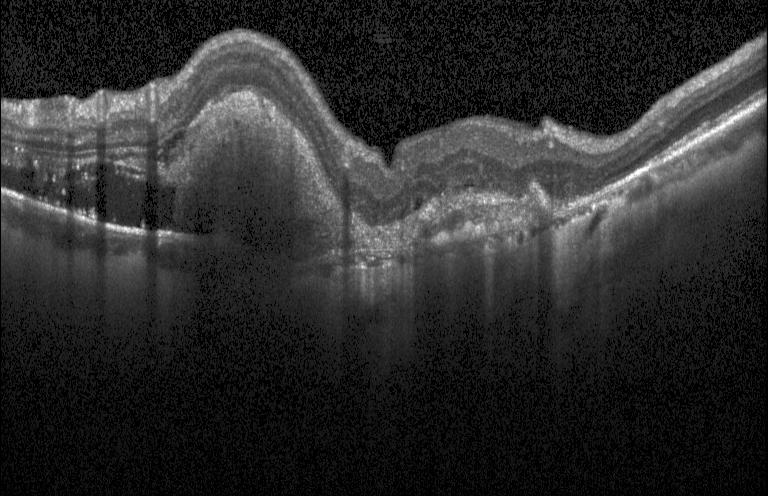 OCT line scan · Heidelberg Spectralis · spectral-domain optical coherence tomography.
Impression: choroidal neovascularization (CNV).